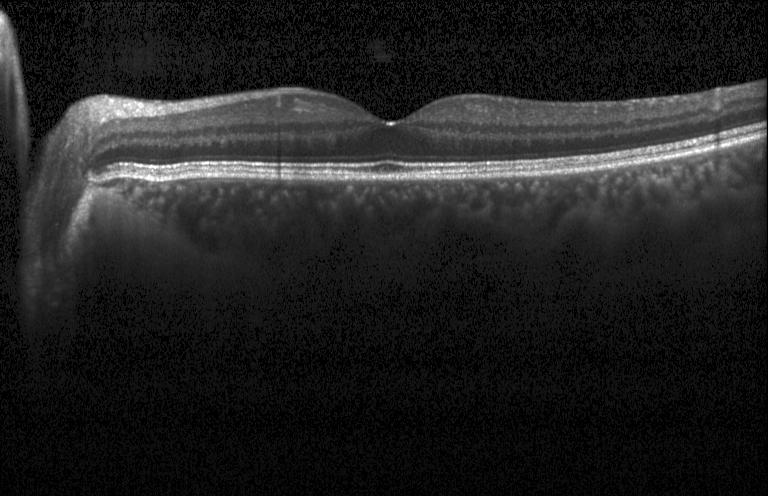 Fovea-centered; Heidelberg Spectralis; optical coherence tomography B-scan; SD-OCT
Assessment: no evidence of choroidal neovascularization, diabetic macular edema, or drusen.